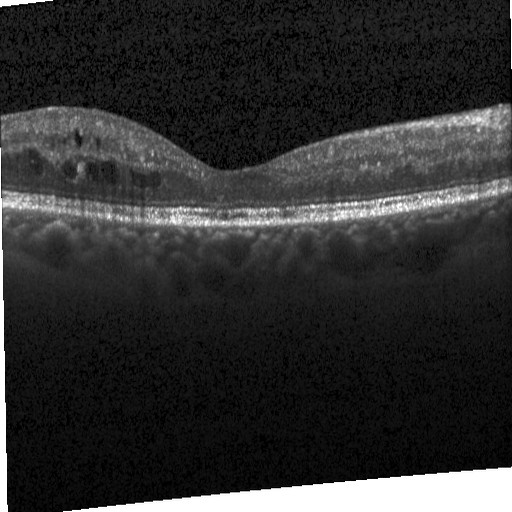 Fovea-centered; SD-OCT; Heidelberg Spectralis OCT system; OCT line scan
Diagnosis: DME.